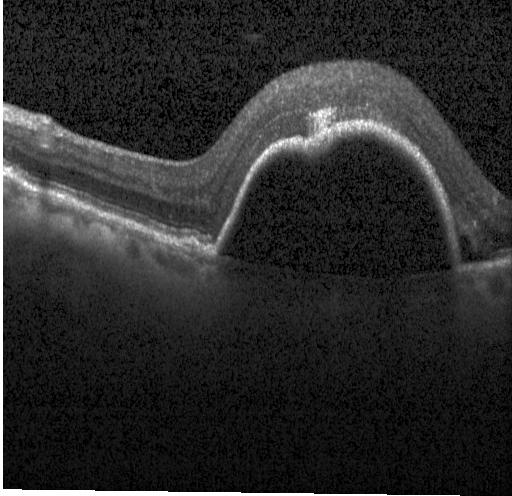

Acquired on a Heidelberg Spectralis; optical coherence tomography B-scan — The scan shows a choroidal neovascular membrane.